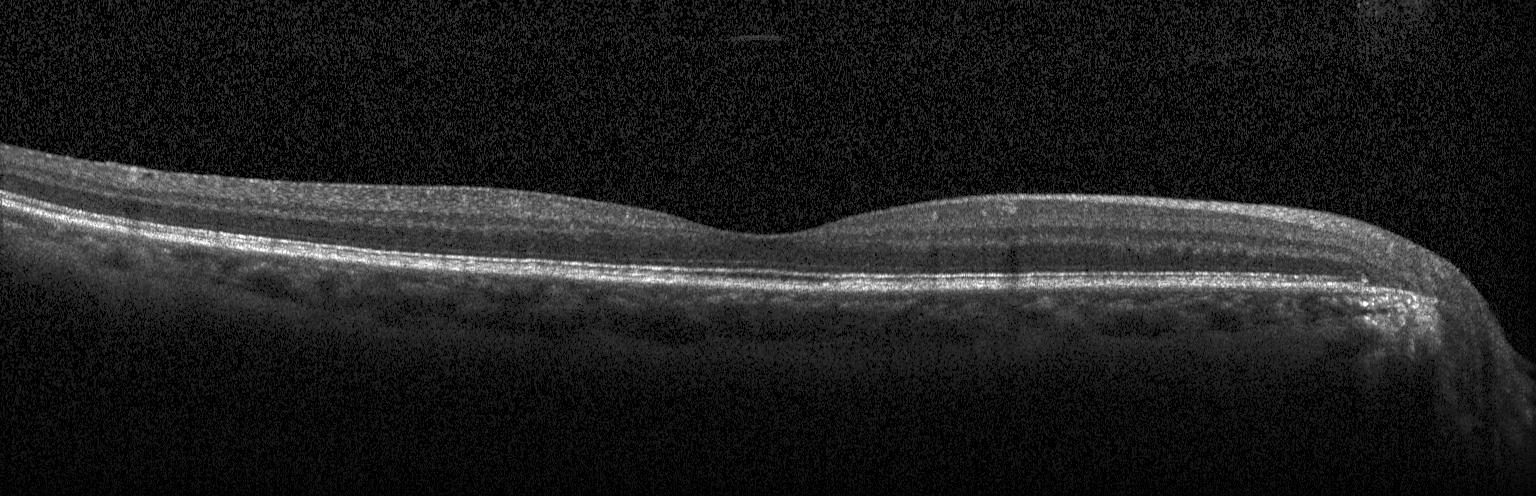
Optical coherence tomography scan
Diagnosis: neither choroidal neovascularization, diabetic macular edema, nor drusen.